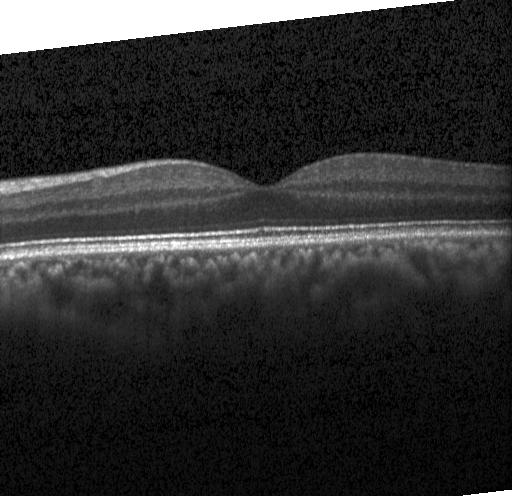

Impression: no choroidal neovascularization, diabetic macular edema, or drusen.